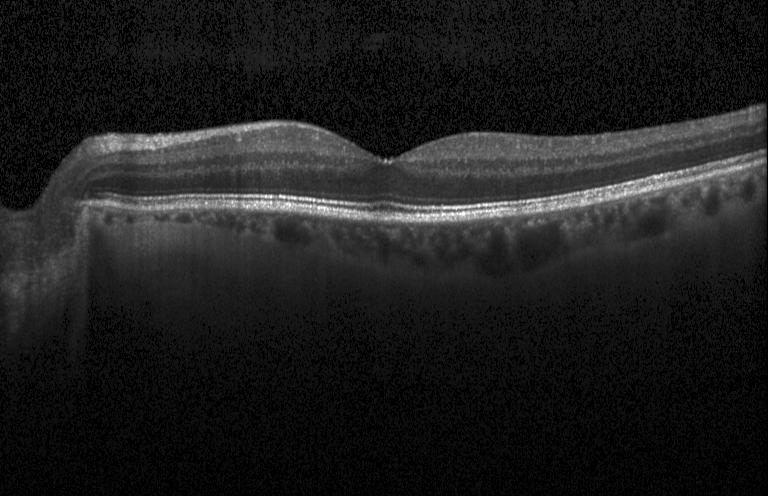

No CNV, DME, or drusen.